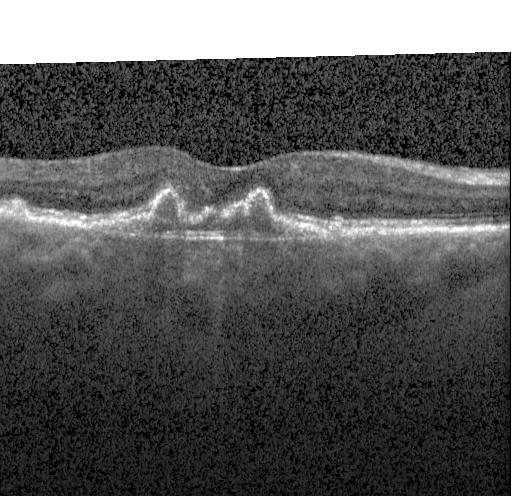
Retinal OCT cross-section. Assessment: CNV.